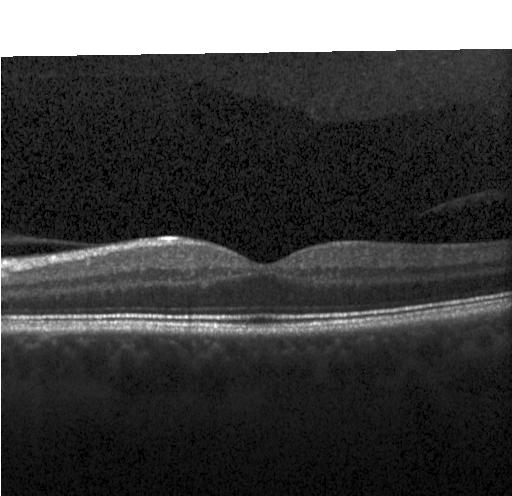

Optical coherence tomography B-scan · Heidelberg Spectralis · macular scan · SD-OCT.
No choroidal neovascularization, no diabetic macular edema, and no drusen.